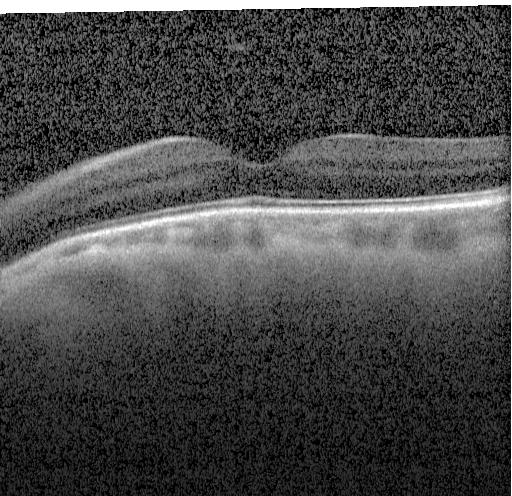 Finding: no evidence of CNV, DME, or drusen.